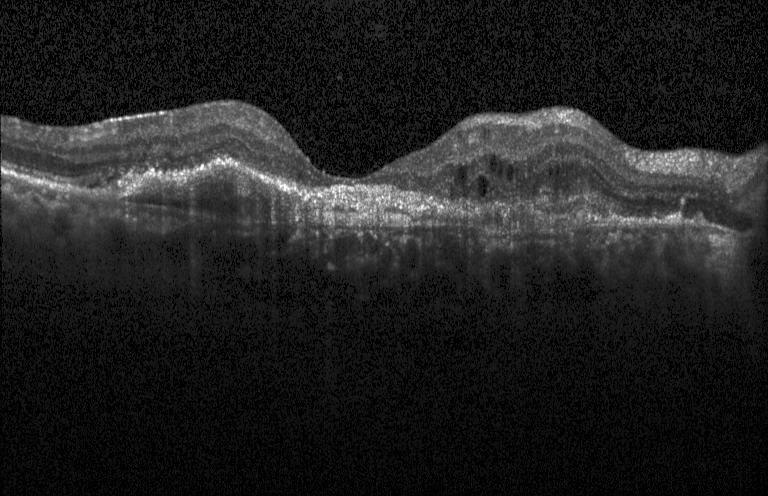

Retinal OCT B-scan. Impression: a choroidal neovascular membrane.